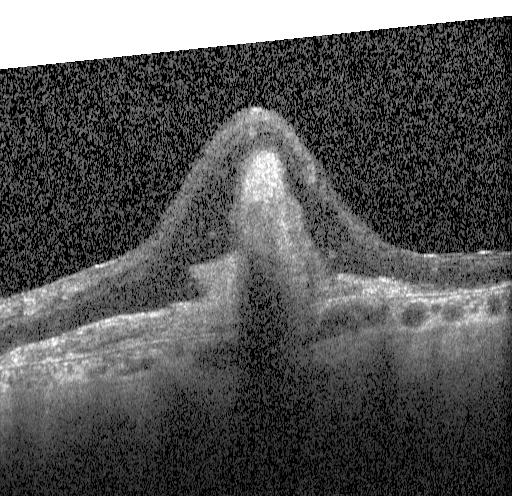

Acquired on a Heidelberg Spectralis. Fovea-centered. OCT B-scan. Spectral-domain optical coherence tomography.
Finding: choroidal neovascularization (CNV).